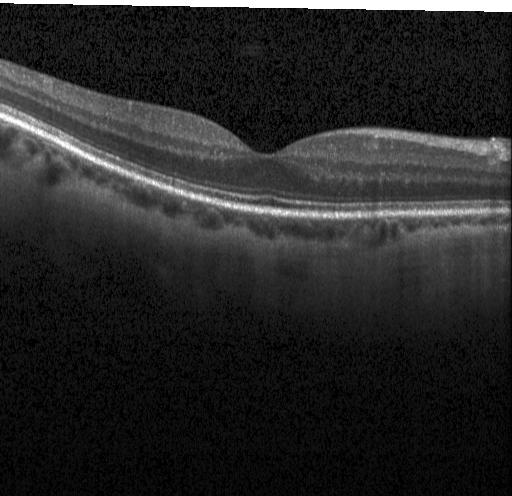 OCT B-scan, spectral-domain optical coherence tomography
Impression: neither choroidal neovascularization, diabetic macular edema, nor drusen.